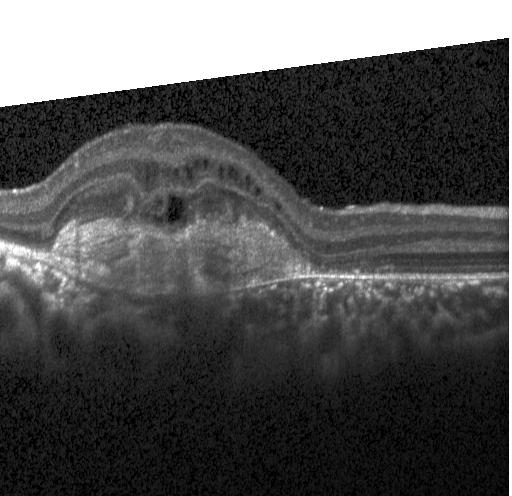
OCT B-scan; spectral-domain OCT — Diagnosis: CNV.